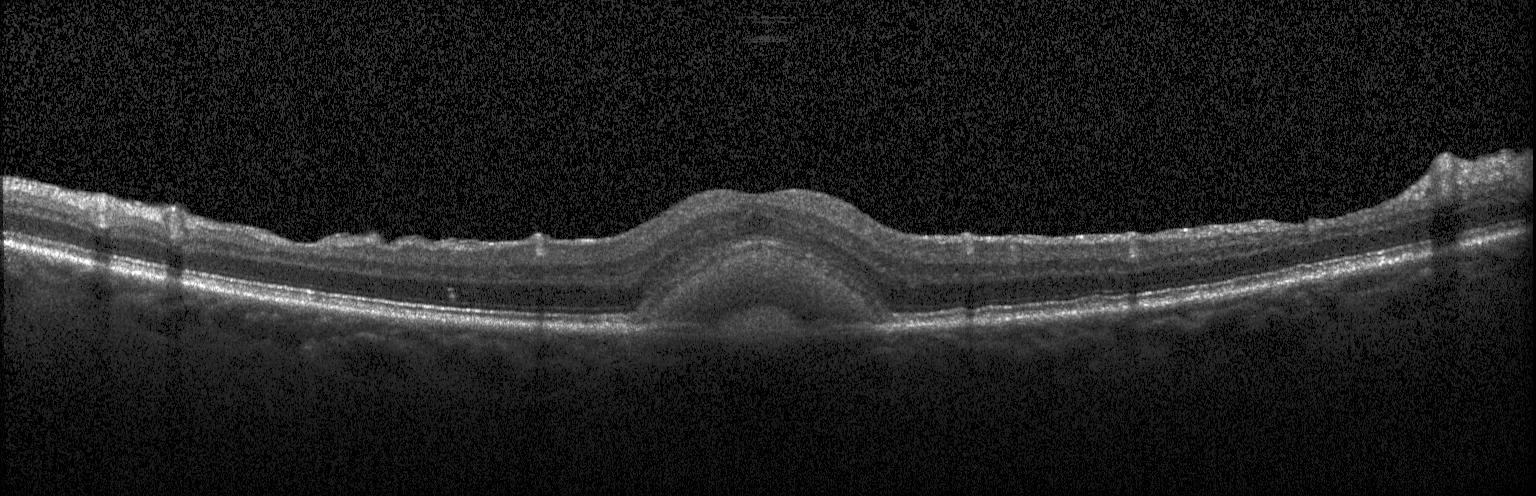
Optical coherence tomography B-scan, Heidelberg Spectralis OCT system. Impression: a choroidal neovascular membrane.